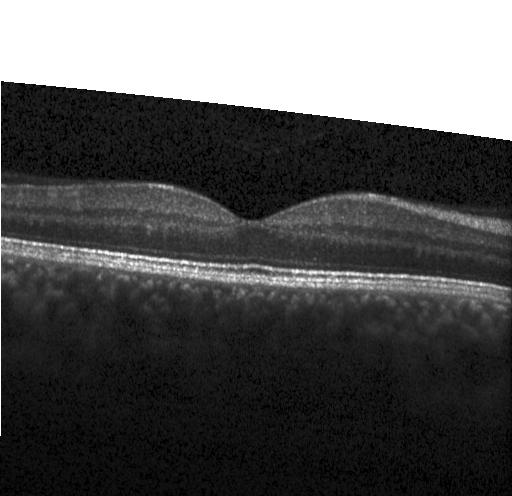

OCT finding: no choroidal neovascularization, no diabetic macular edema, and no drusen.